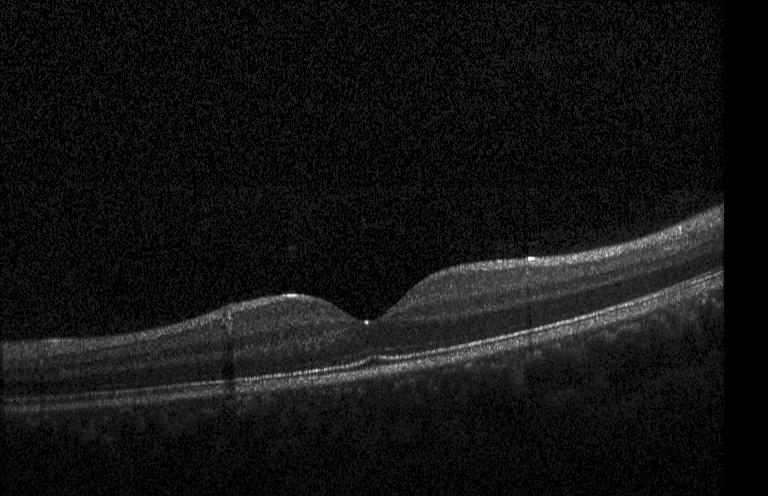
Centered on the fovea, Heidelberg Spectralis, optical coherence tomography B-scan, SD-OCT. This B-scan demonstrates no evidence of choroidal neovascularization, diabetic macular edema, or drusen.